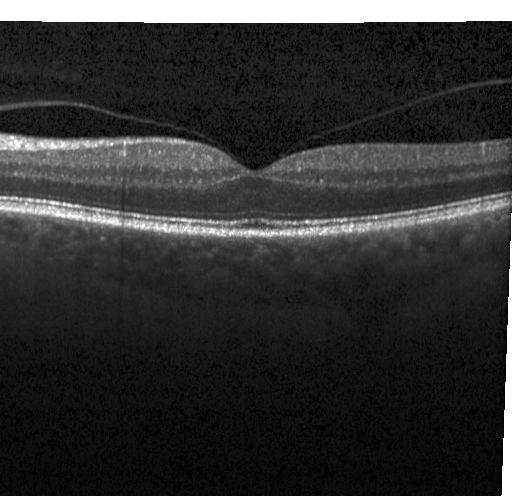
OCT line scan. Acquired on a Heidelberg Spectralis
Diagnosis: neither choroidal neovascularization, diabetic macular edema, nor drusen.